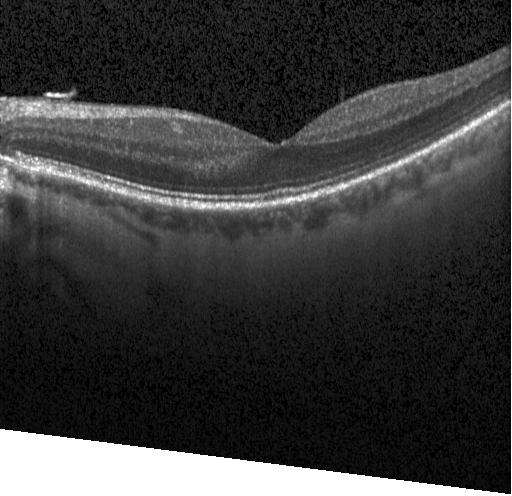

OCT B-scan · Heidelberg Spectralis OCT system · through the macula.
Diagnosis: neither choroidal neovascularization, diabetic macular edema, nor drusen.